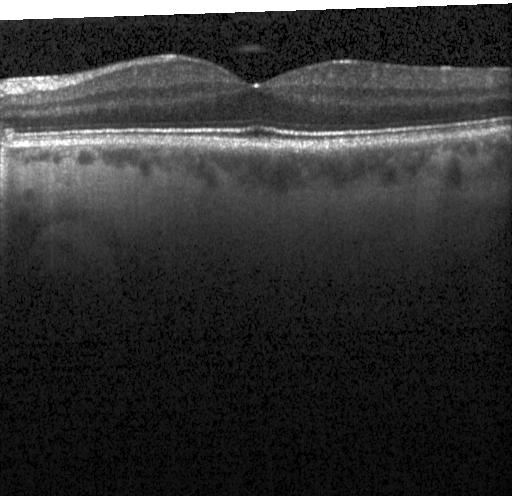
Optical coherence tomography scan — OCT finding: no choroidal neovascularization, no diabetic macular edema, and no drusen.